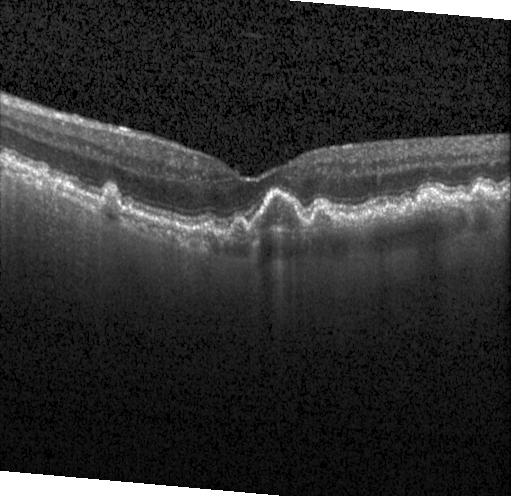

OCT finding: drusen.